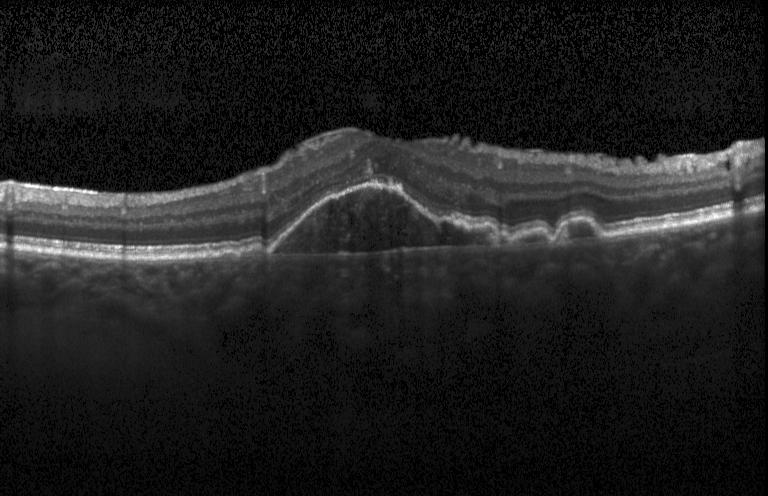

Retinal OCT B-scan
Finding: choroidal neovascularization (CNV).